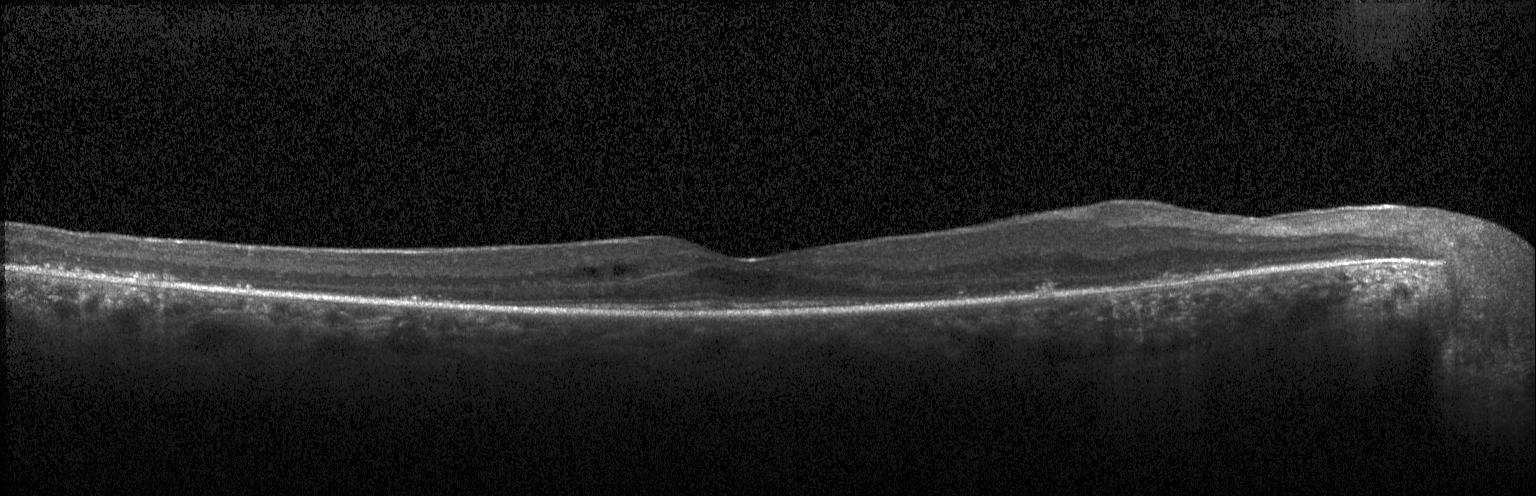

Spectral-domain OCT. Through the macula. OCT line scan
Dx: DME.